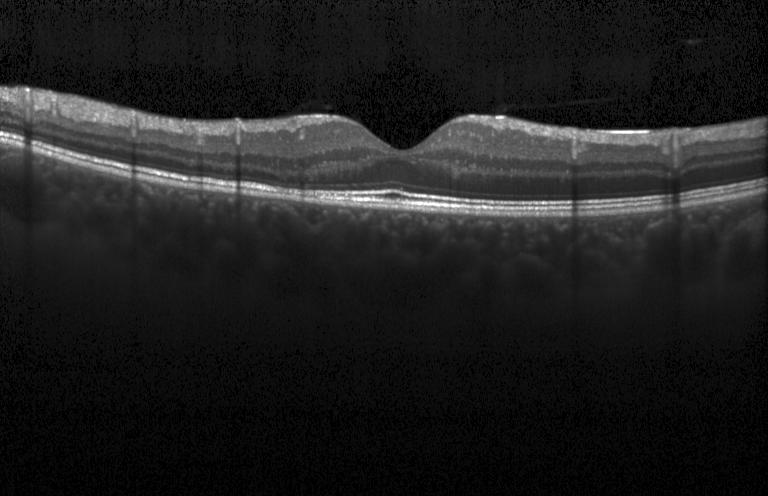

Instrument: Heidelberg Spectralis; OCT line scan; SD-OCT; centered on the fovea.
Diagnosis: neither choroidal neovascularization, diabetic macular edema, nor drusen.